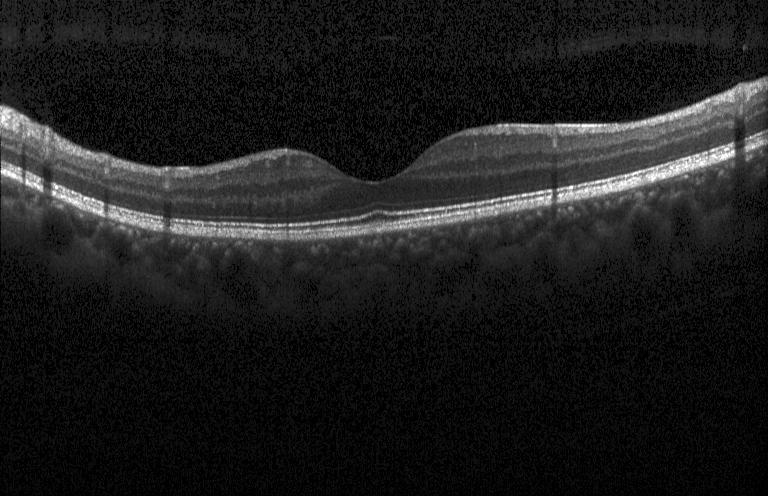

Optical coherence tomography B-scan · Heidelberg Spectralis. This B-scan demonstrates neither CNV, DME, nor drusen.